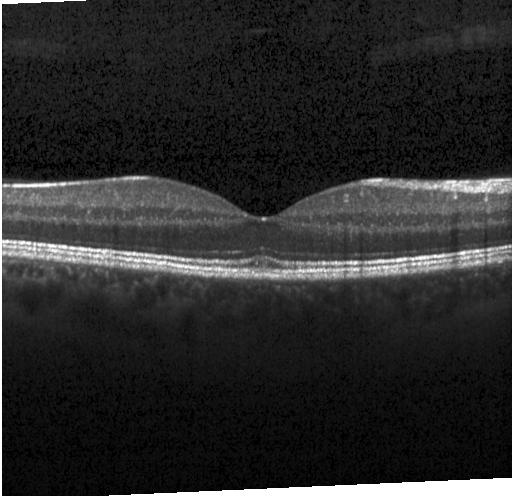 Spectral-domain optical coherence tomography. OCT B-scan.
Impression: no choroidal neovascularization, diabetic macular edema, or drusen.